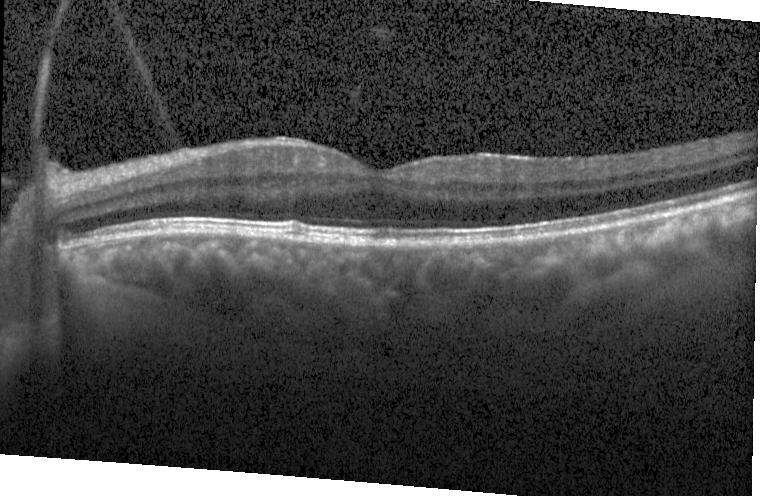 Retinal OCT cross-section showing no evidence of choroidal neovascularization, diabetic macular edema, or drusen.